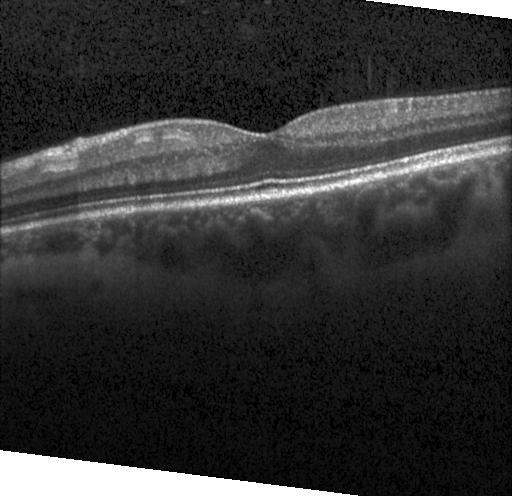
Optical coherence tomography B-scan. Spectral-domain OCT. Fovea-centered. Heidelberg Spectralis OCT system.
No choroidal neovascularization, diabetic macular edema, or drusen.